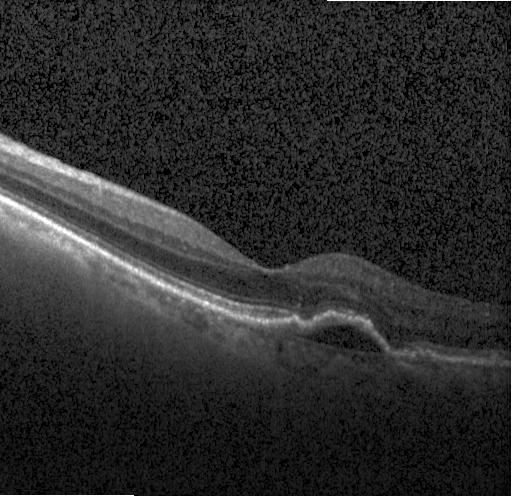
Heidelberg Spectralis · optical coherence tomography B-scan. Diagnosis: choroidal neovascularization.